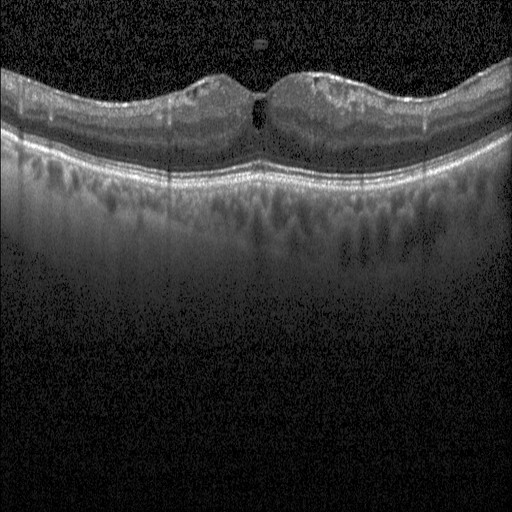
Retinal OCT B-scan; instrument: Heidelberg Spectralis; horizontal scan through the fovea; SD-OCT.
Impression: DME.